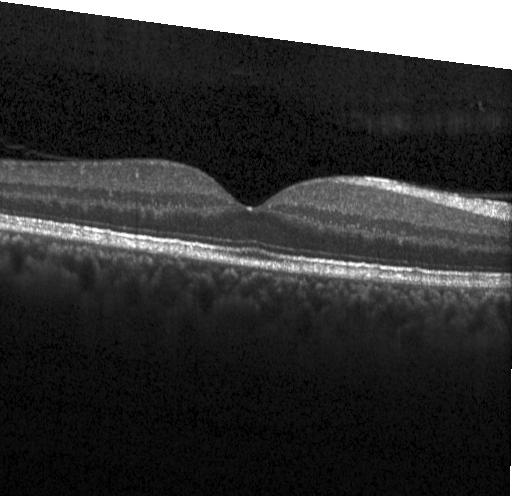 Macular OCT: no CNV, no DME, and no drusen.